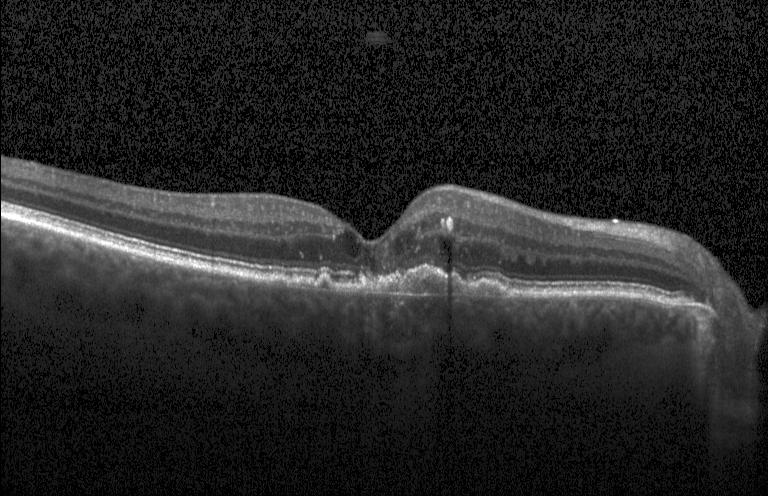 OCT finding: choroidal neovascularization (CNV).